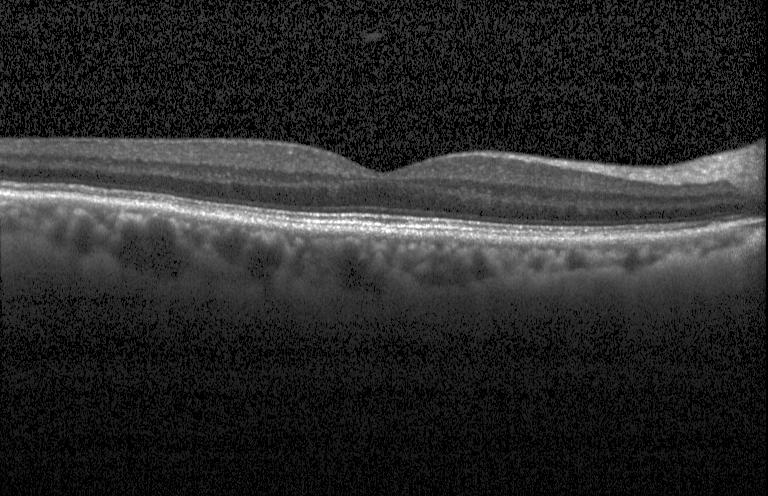

OCT B-scan showing neither CNV, DME, nor drusen.